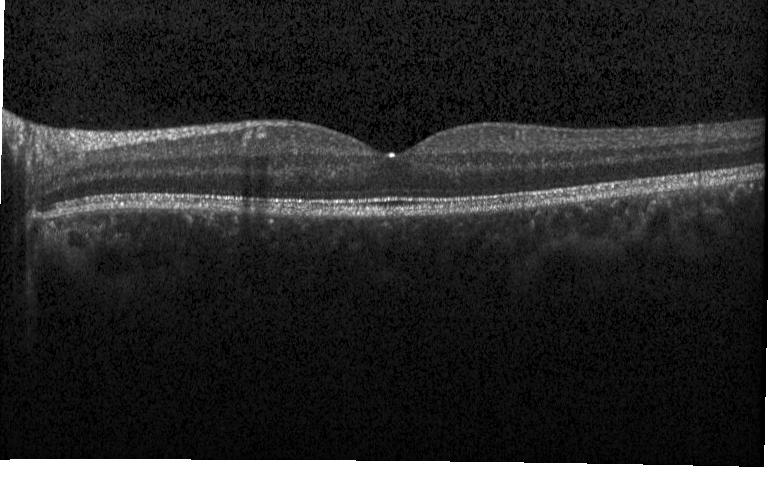 Heidelberg Spectralis, retinal OCT B-scan, spectral-domain optical coherence tomography — Macular OCT: no evidence of CNV, DME, or drusen.